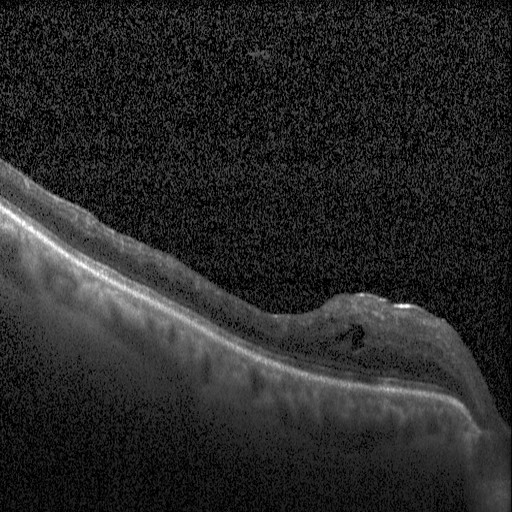 OCT line scan. Diabetic macular edema.